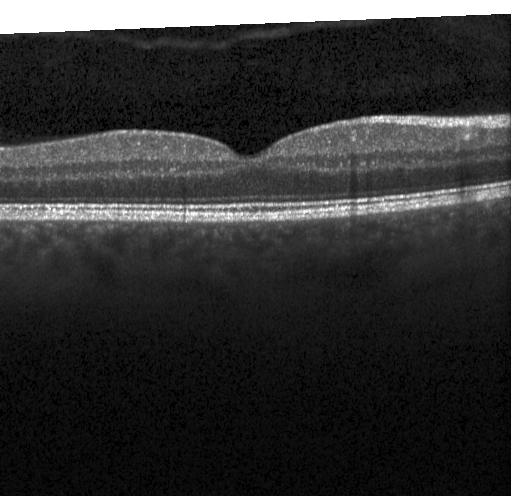
Impression: no choroidal neovascularization, no diabetic macular edema, and no drusen.